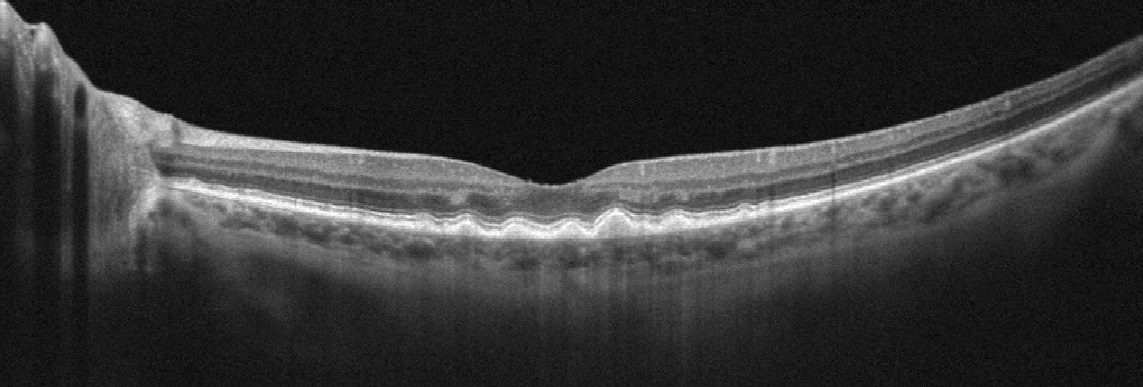
Diagnosis: age-related macular degeneration.